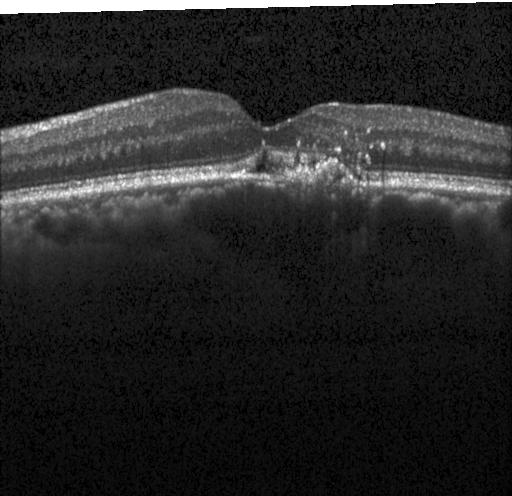
Centered on the fovea · OCT line scan
Dx: a choroidal neovascular membrane.